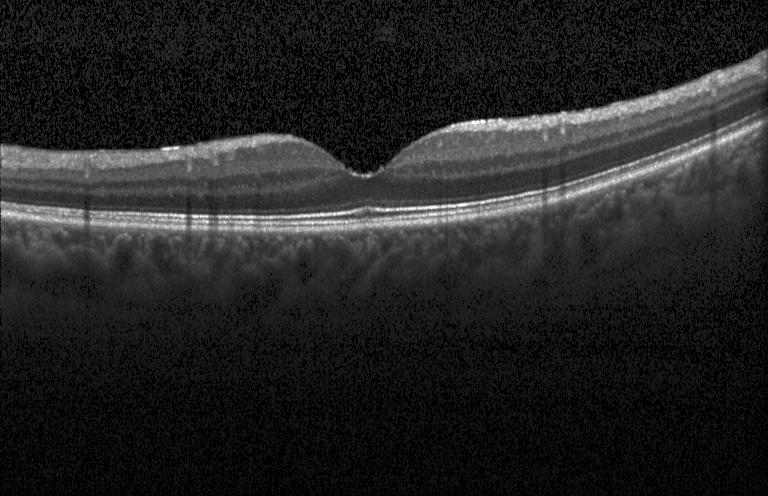
Optical coherence tomography scan; instrument: Heidelberg Spectralis — The scan shows neither CNV, DME, nor drusen.